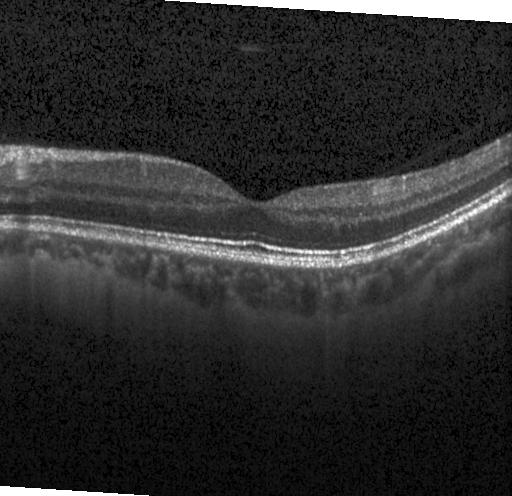

Diagnosis: neither choroidal neovascularization, diabetic macular edema, nor drusen.